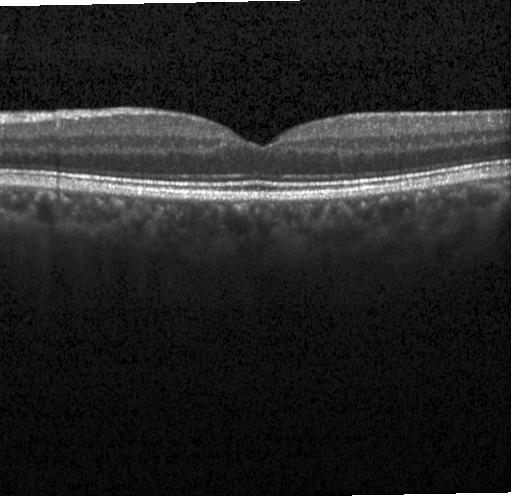

Macular scan, instrument: Heidelberg Spectralis, OCT B-scan.
OCT finding: no evidence of choroidal neovascularization, diabetic macular edema, or drusen.